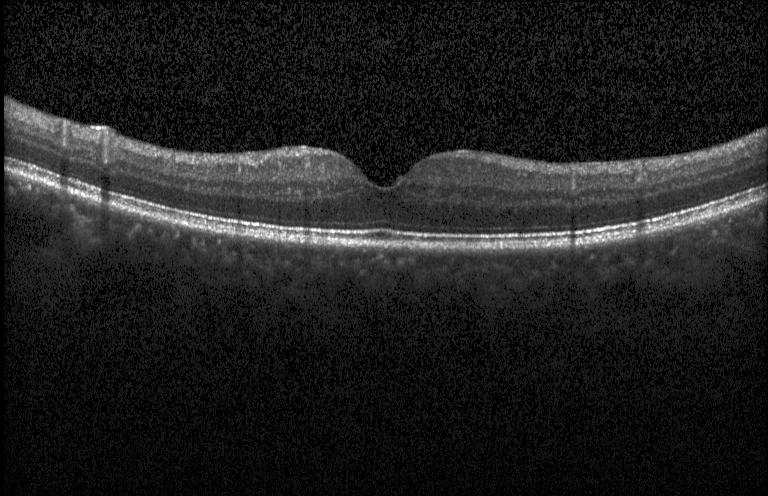
OCT scan showing no evidence of choroidal neovascularization, diabetic macular edema, or drusen.